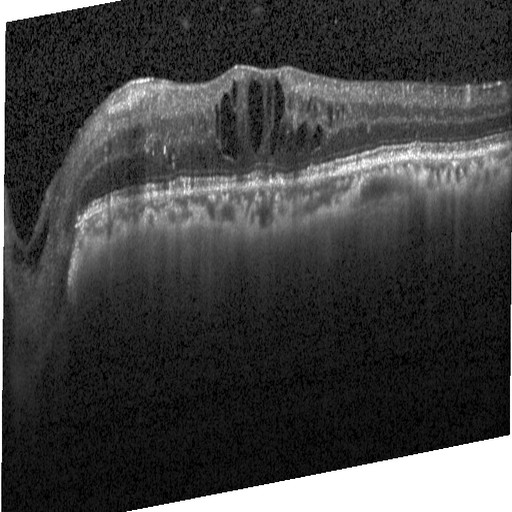
Retinal OCT B-scan. Diagnosis: diabetic macular edema.